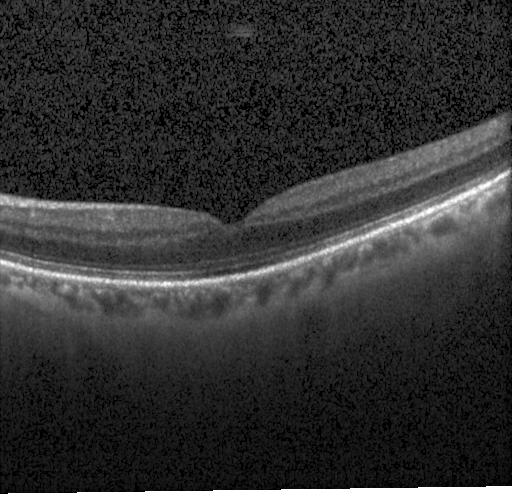

Retinal OCT cross-section. Centered on the fovea. Instrument: Heidelberg Spectralis. SD-OCT.
Impression: no evidence of choroidal neovascularization, diabetic macular edema, or drusen.